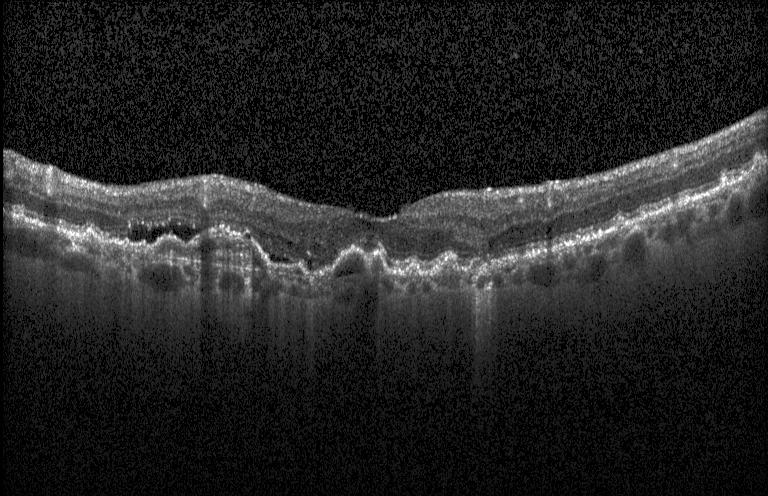 Optical coherence tomography B-scan. Spectral-domain OCT. Macular scan. Assessment: choroidal neovascularization.